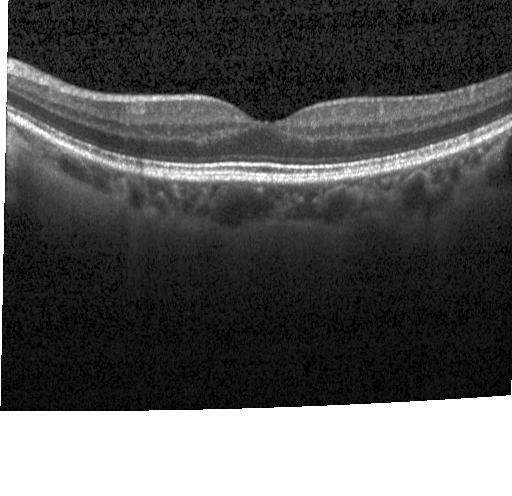
OCT B-scan showing neither choroidal neovascularization, diabetic macular edema, nor drusen.